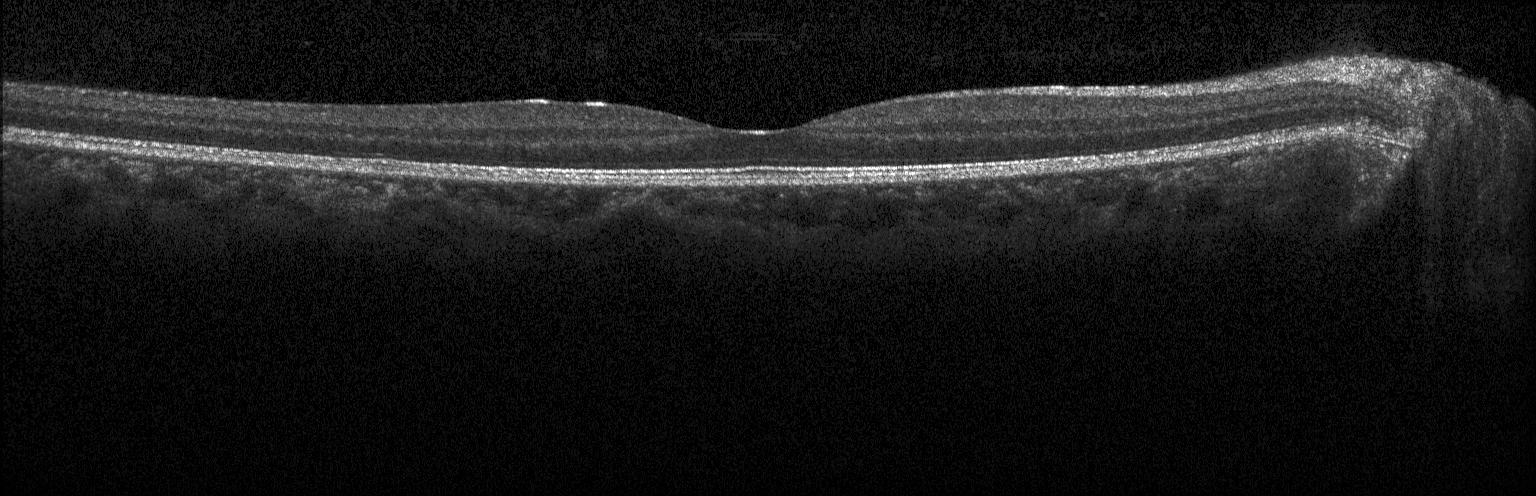 Retinal OCT B-scan — This B-scan demonstrates no choroidal neovascularization, diabetic macular edema, or drusen.